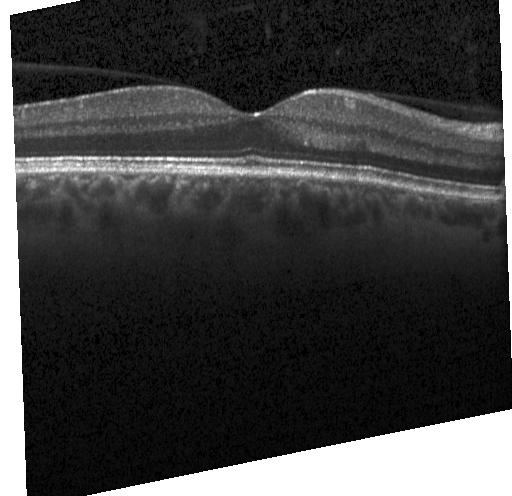 Optical coherence tomography B-scan; spectral-domain optical coherence tomography — Macular OCT: no evidence of choroidal neovascularization, diabetic macular edema, or drusen.